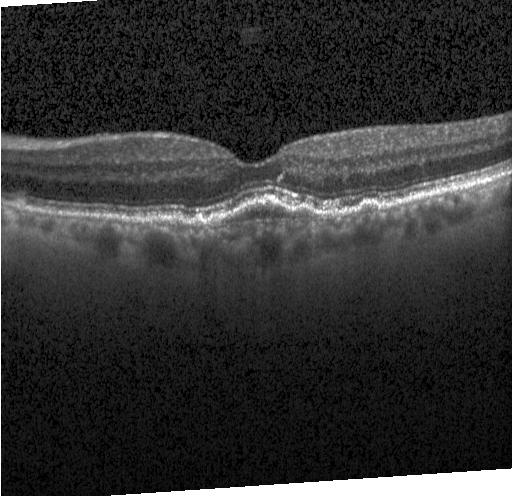 Optical coherence tomography scan
The scan shows a choroidal neovascular membrane.